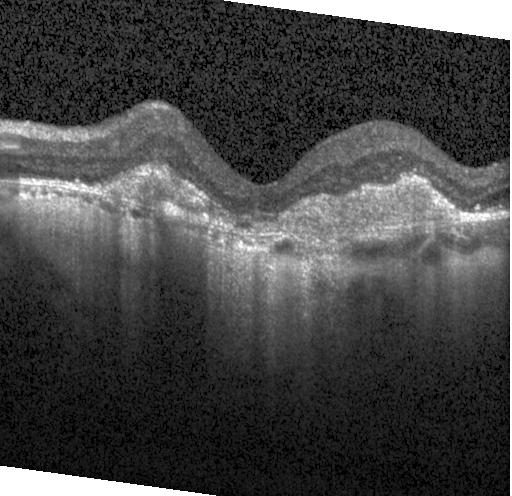

OCT B-scan — Finding: choroidal neovascularization (CNV).